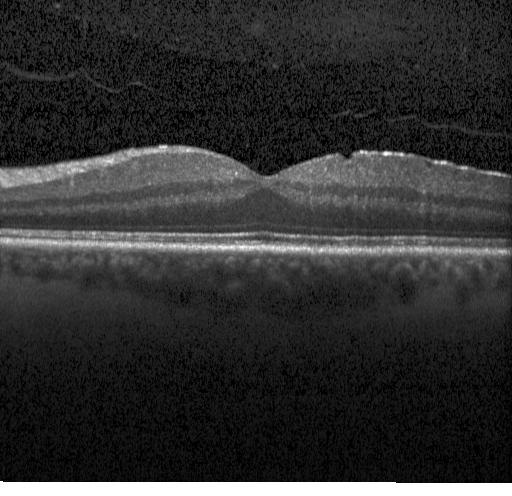
Spectral-domain OCT B-scan: no CNV, no DME, and no drusen.